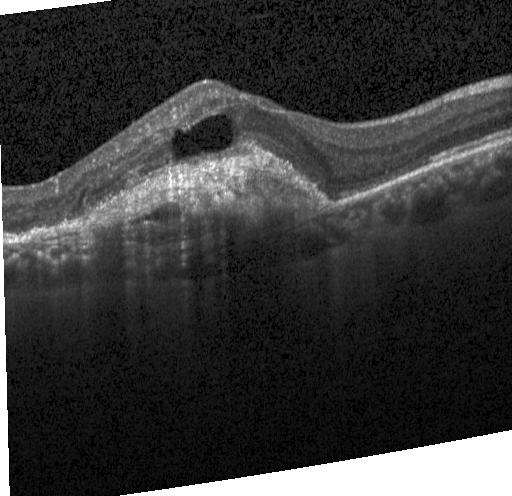

Macular OCT: a choroidal neovascular membrane.